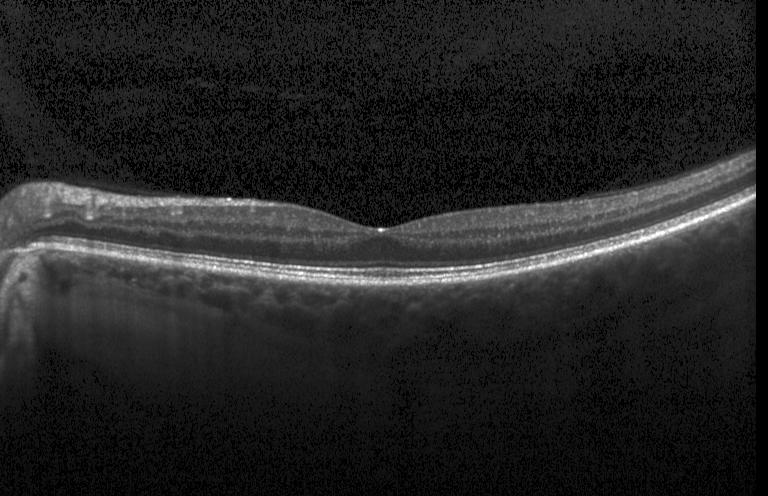

Heidelberg Spectralis OCT system, centered on the fovea, spectral-domain optical coherence tomography, retinal OCT B-scan.
Neither choroidal neovascularization, diabetic macular edema, nor drusen.